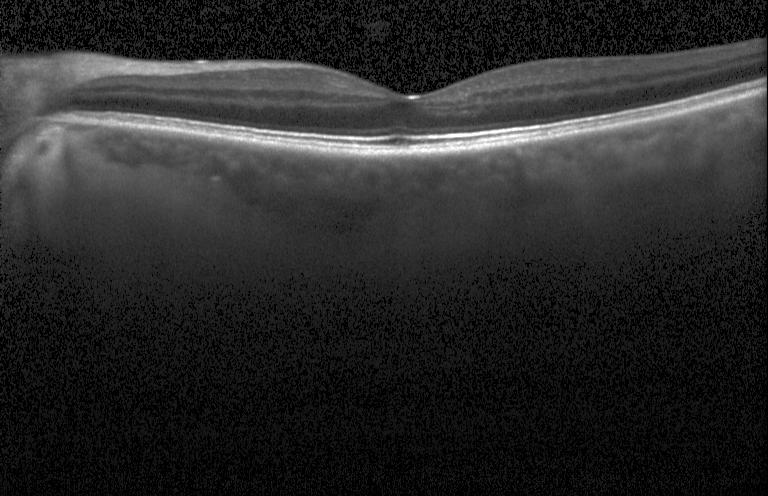
Macular OCT: neither choroidal neovascularization, diabetic macular edema, nor drusen.